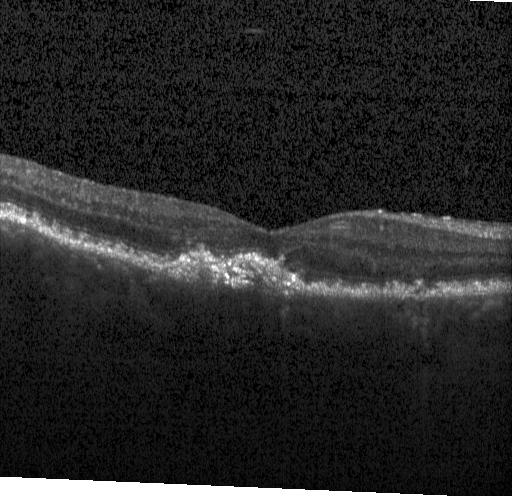

SD-OCT · retinal OCT B-scan
This B-scan demonstrates choroidal neovascularization.